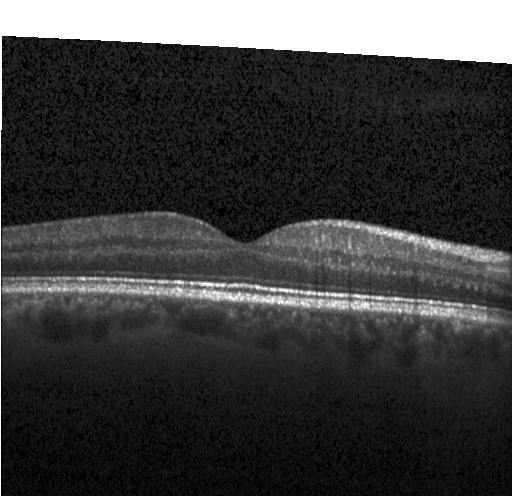

Spectral-domain OCT, optical coherence tomography B-scan.
This B-scan demonstrates no evidence of CNV, DME, or drusen.